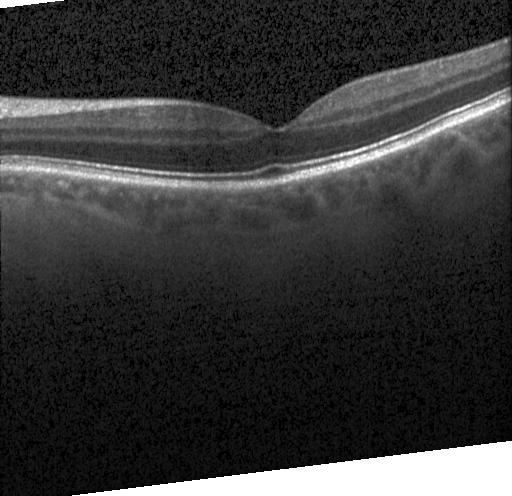 Optical coherence tomography B-scan — No CNV, no DME, and no drusen.